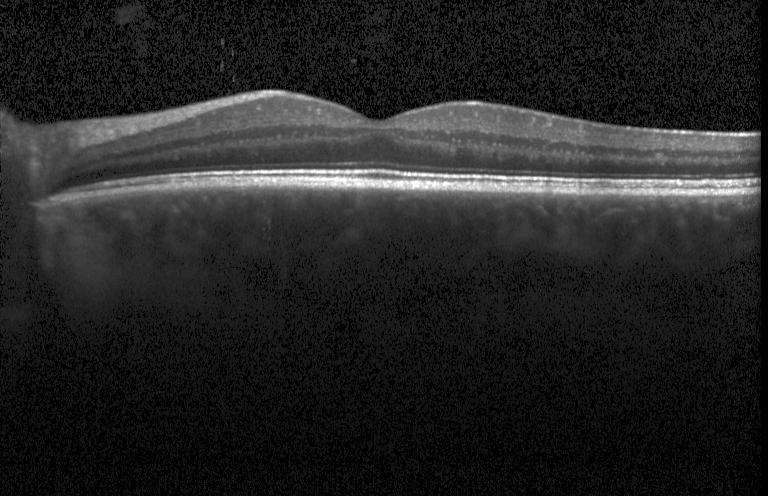

OCT B-scan showing no evidence of choroidal neovascularization, diabetic macular edema, or drusen.